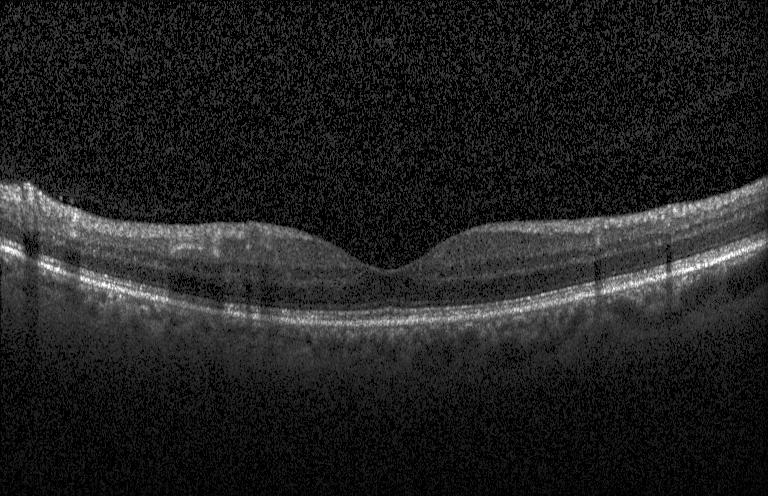

Heidelberg Spectralis OCT system. Retinal OCT B-scan. SD-OCT. Fovea-centered.
Assessment: no evidence of choroidal neovascularization, diabetic macular edema, or drusen.